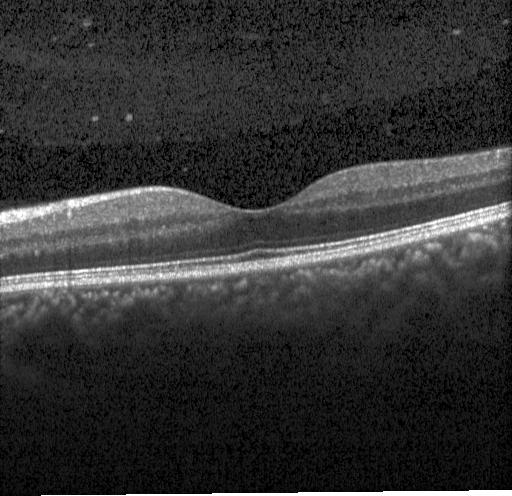

Optical coherence tomography scan
Finding: no evidence of choroidal neovascularization, diabetic macular edema, or drusen.